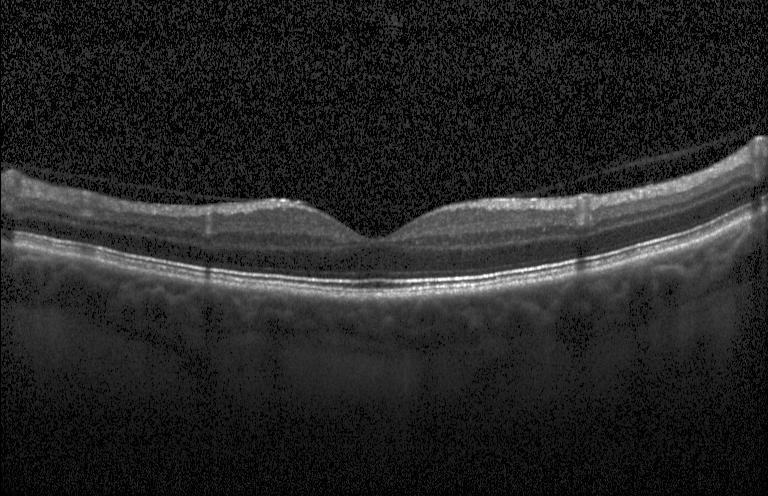 Finding: no evidence of choroidal neovascularization, diabetic macular edema, or drusen.